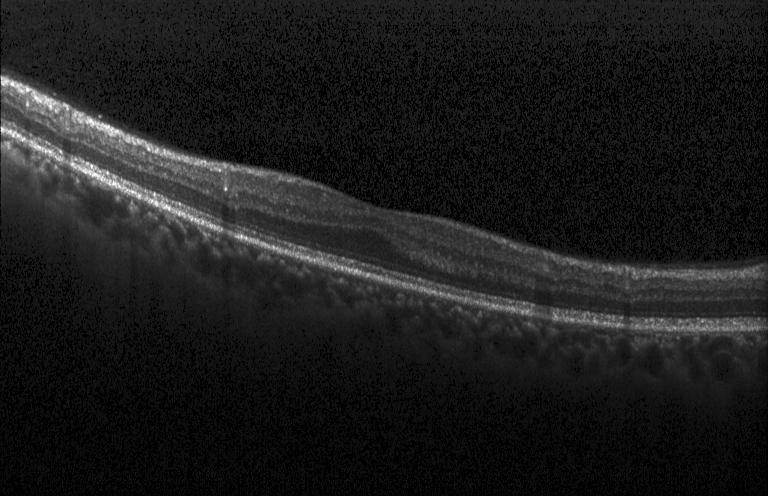
Finding: no evidence of CNV, DME, or drusen.